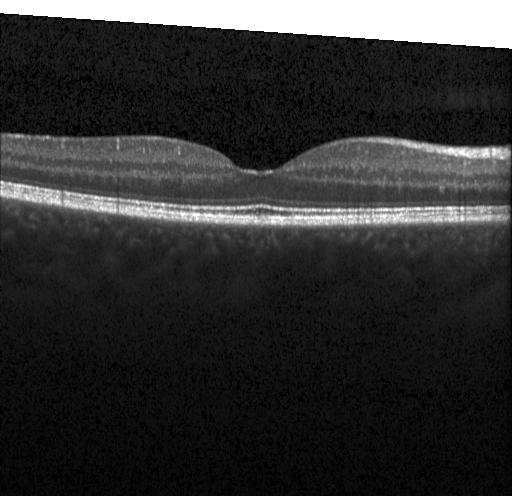
Retinal OCT B-scan
Finding: neither CNV, DME, nor drusen.